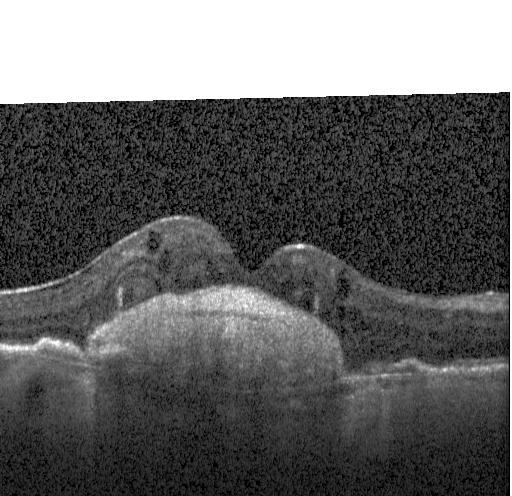
OCT B-scan showing a choroidal neovascular membrane.